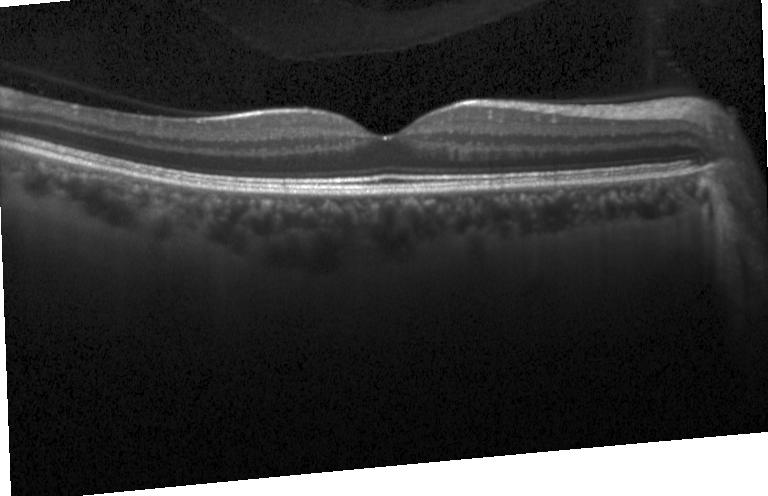 Optical coherence tomography B-scan — Finding: no choroidal neovascularization, diabetic macular edema, or drusen.